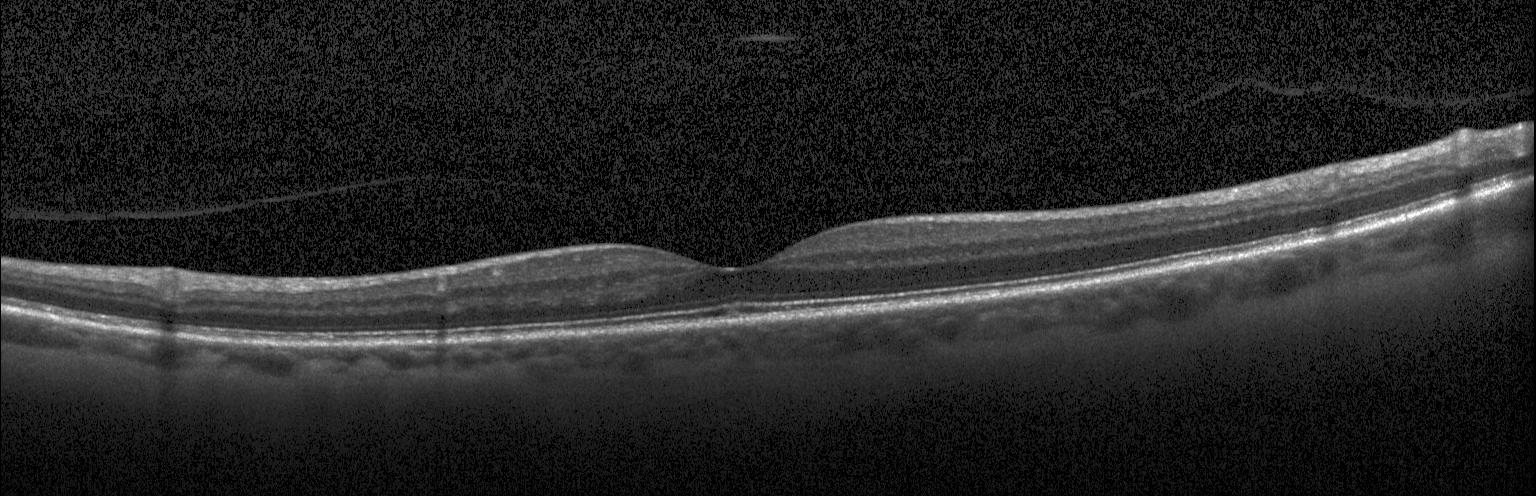

Fovea-centered · acquired on a Heidelberg Spectralis · optical coherence tomography B-scan · spectral-domain optical coherence tomography.
Neither CNV, DME, nor drusen.